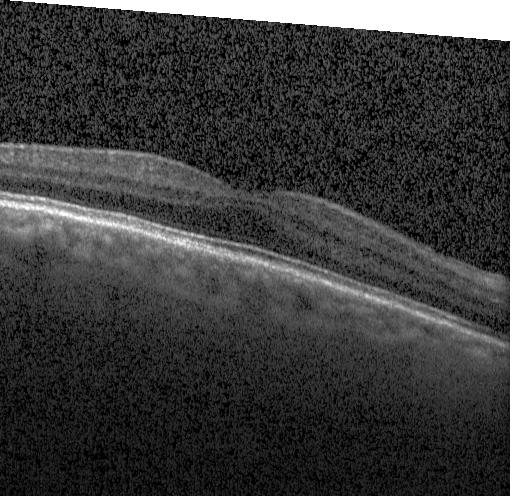

SD-OCT · horizontal scan through the fovea · OCT B-scan — Assessment: no choroidal neovascularization, no diabetic macular edema, and no drusen.